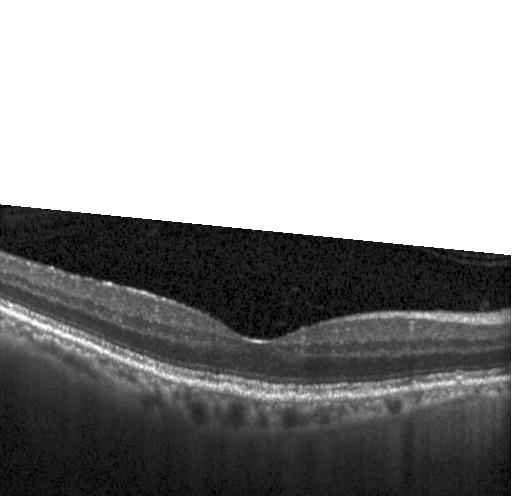

OCT line scan · Heidelberg Spectralis — Assessment: no choroidal neovascularization, diabetic macular edema, or drusen.